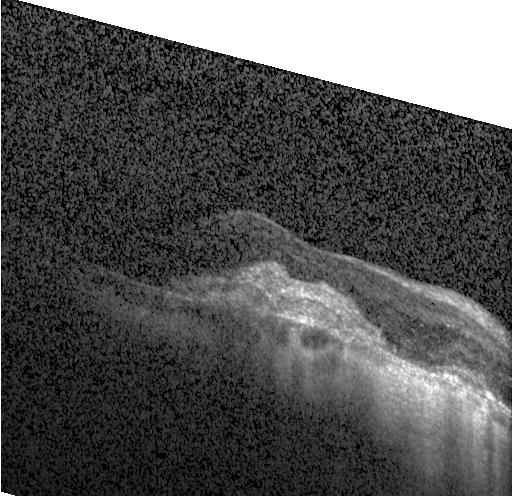 OCT line scan; spectral-domain optical coherence tomography.
Macular OCT: CNV.